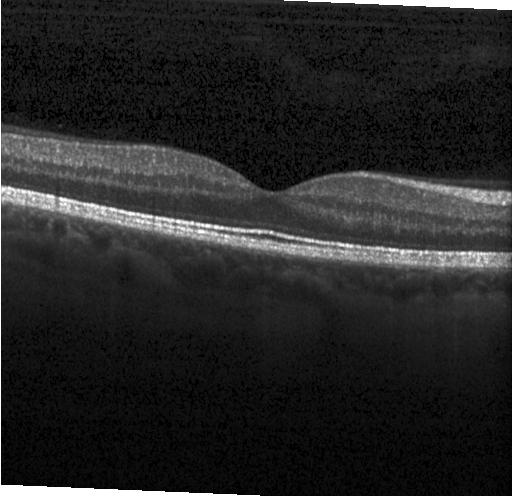
OCT B-scan.
Assessment: no choroidal neovascularization, no diabetic macular edema, and no drusen.